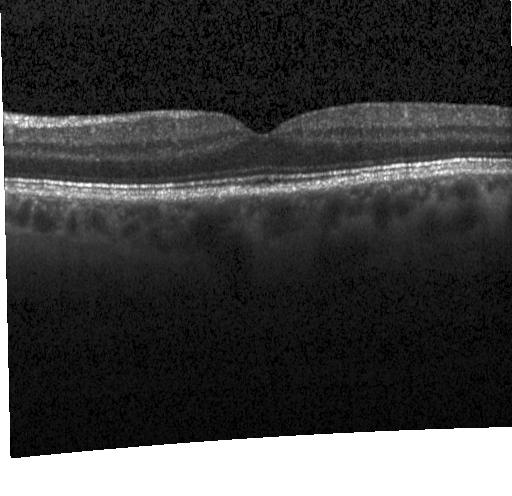 Diagnosis: no choroidal neovascularization, no diabetic macular edema, and no drusen.